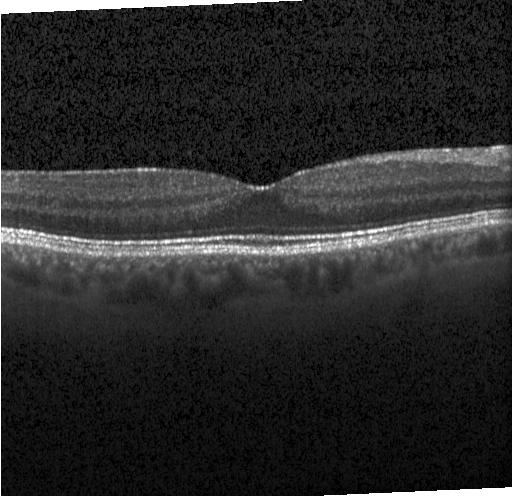
Acquired on a Heidelberg Spectralis · OCT line scan · macular scan — This B-scan demonstrates no choroidal neovascularization, diabetic macular edema, or drusen.